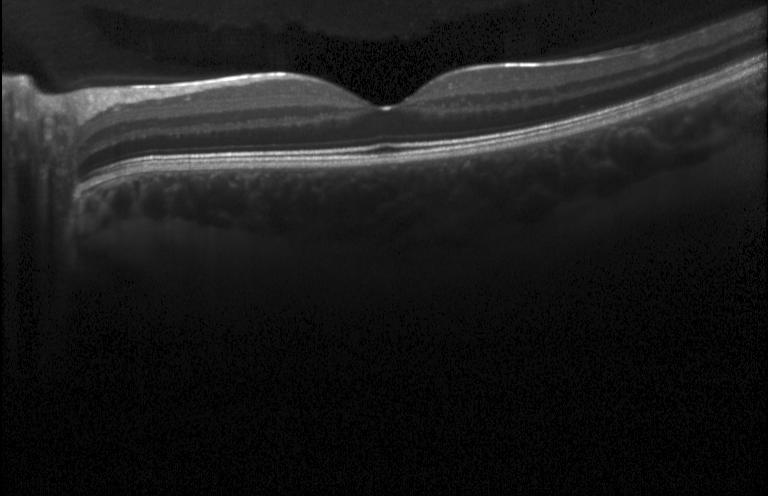
Optical coherence tomography B-scan; spectral-domain OCT; instrument: Heidelberg Spectralis.
Diagnosis: no CNV, DME, or drusen.